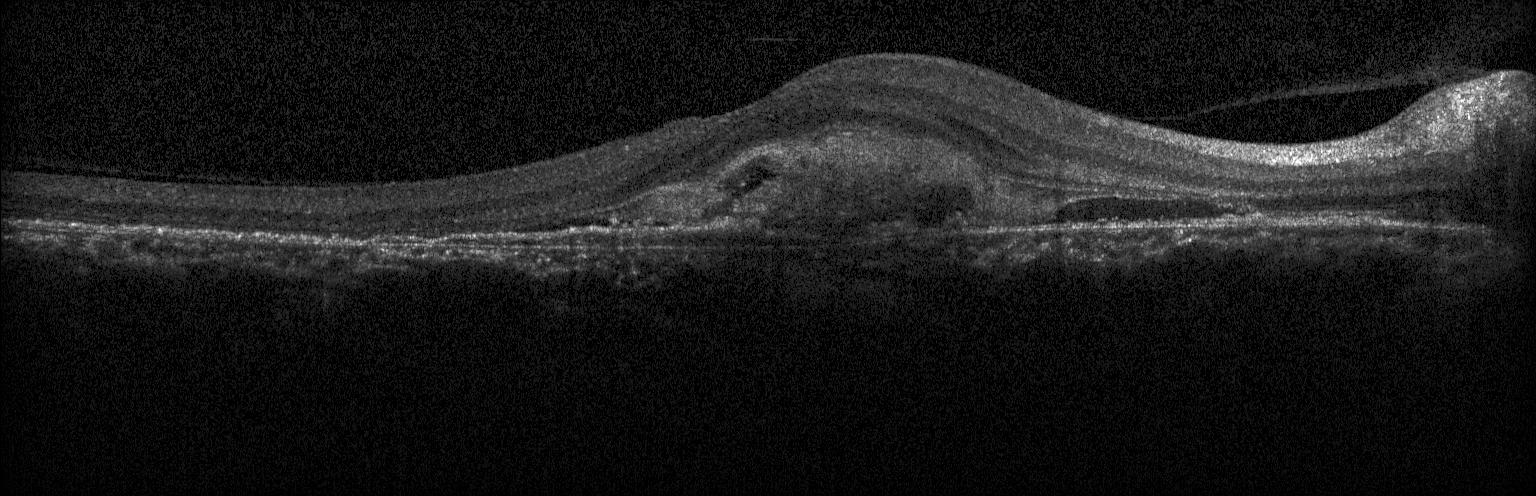 OCT B-scan showing choroidal neovascularization (CNV).